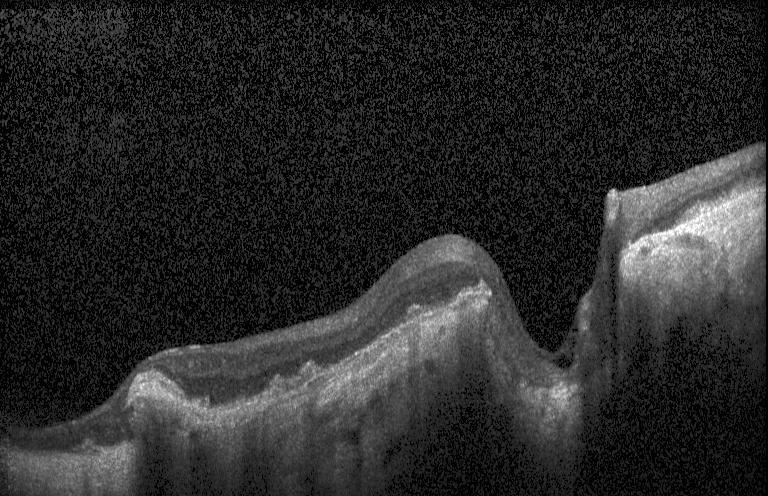

OCT line scan · SD-OCT · macular scan · acquired on a Heidelberg Spectralis
OCT finding: a choroidal neovascular membrane.